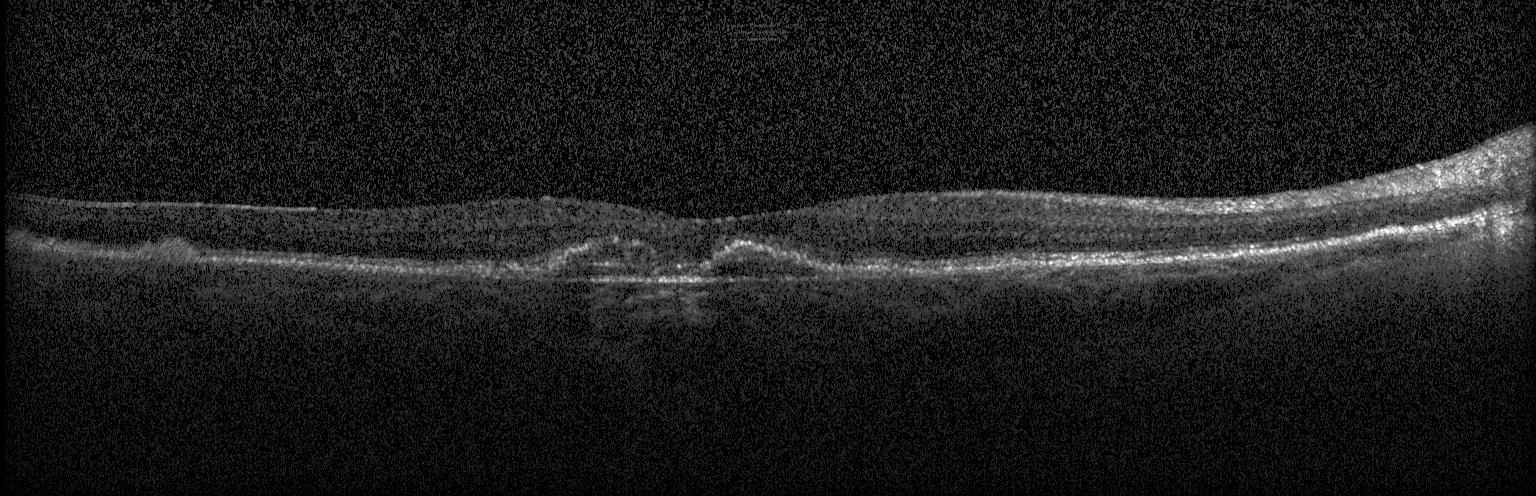

Choroidal neovascularization.